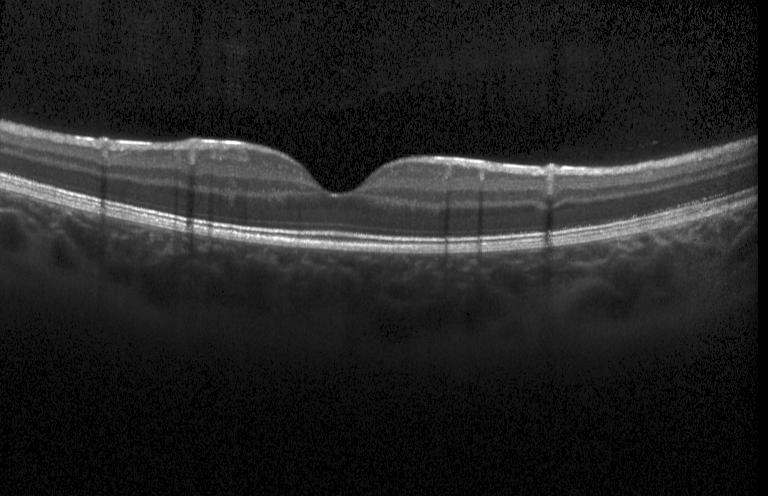

OCT B-scan showing no choroidal neovascularization, no diabetic macular edema, and no drusen.